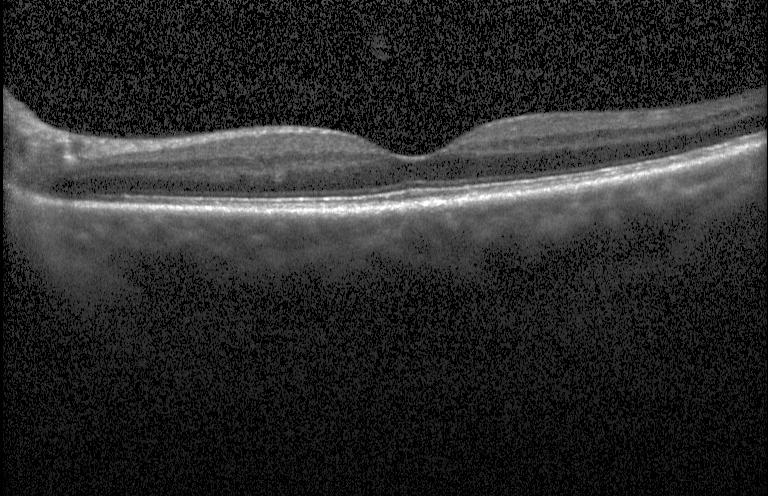
Optical coherence tomography scan — Impression: no CNV, no DME, and no drusen.